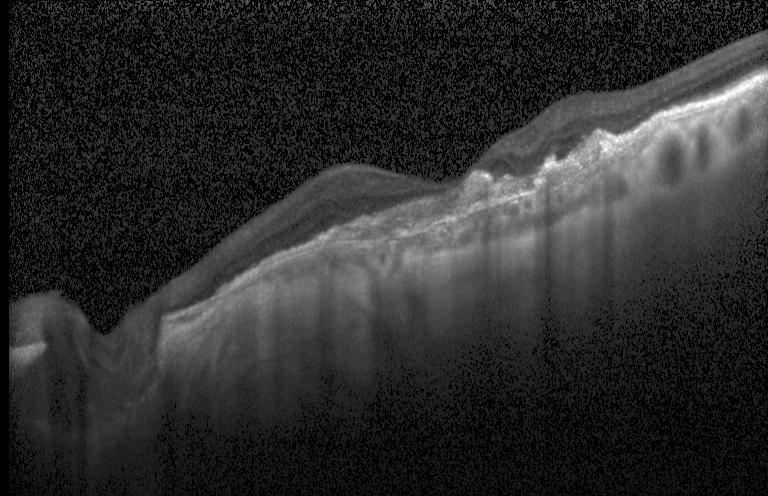

OCT scan showing choroidal neovascularization (CNV).